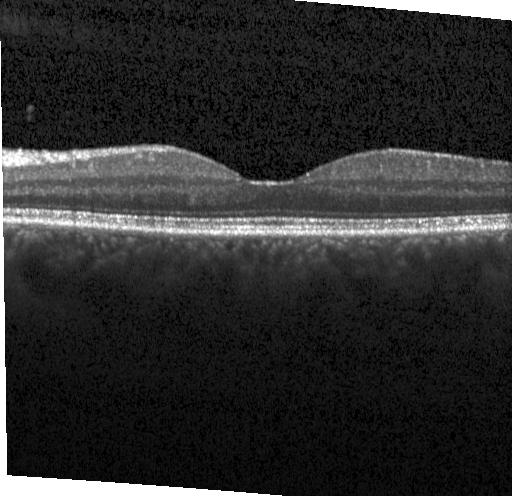 Fovea-centered · retinal OCT B-scan · instrument: Heidelberg Spectralis — The scan shows no choroidal neovascularization, diabetic macular edema, or drusen.